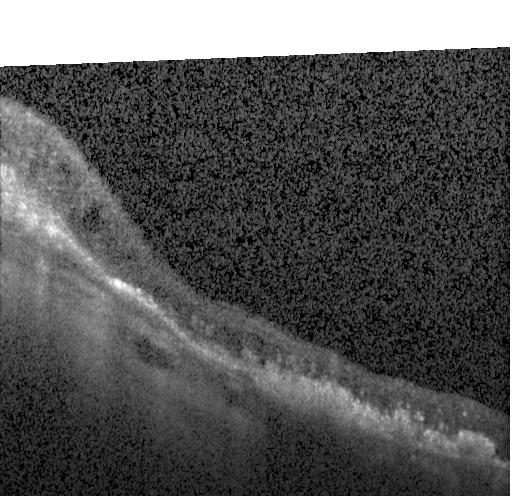 Dx: a choroidal neovascular membrane.